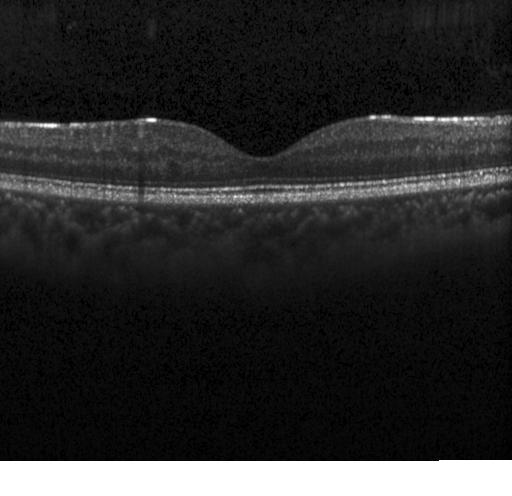
OCT line scan; Heidelberg Spectralis OCT system
The scan shows no CNV, DME, or drusen.